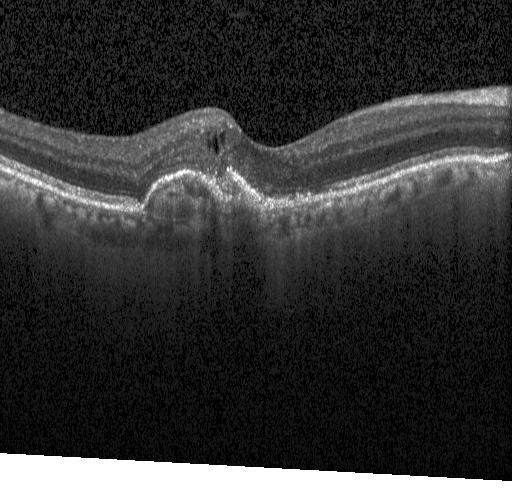

Fovea-centered · Heidelberg Spectralis · retinal OCT B-scan · spectral-domain OCT — Impression: choroidal neovascularization (CNV).